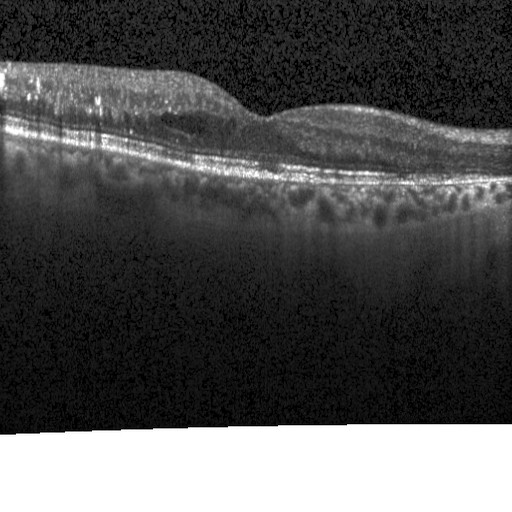
OCT line scan · centered on the fovea · SD-OCT. OCT finding: diabetic macular edema (DME).